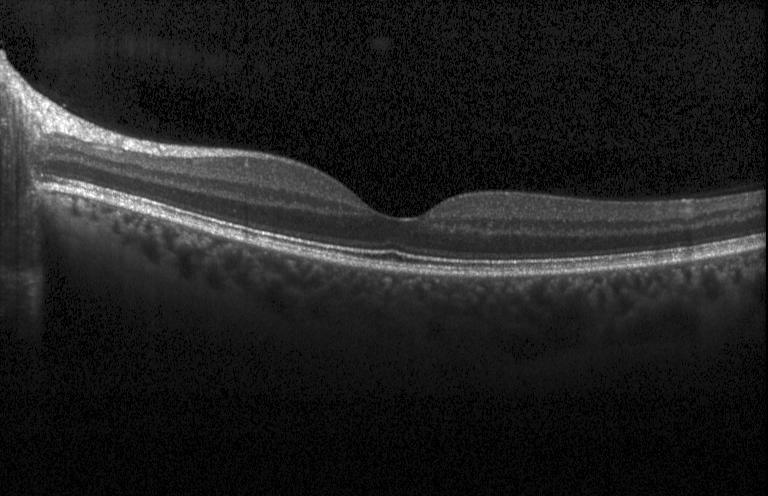
Dx: no choroidal neovascularization, no diabetic macular edema, and no drusen.